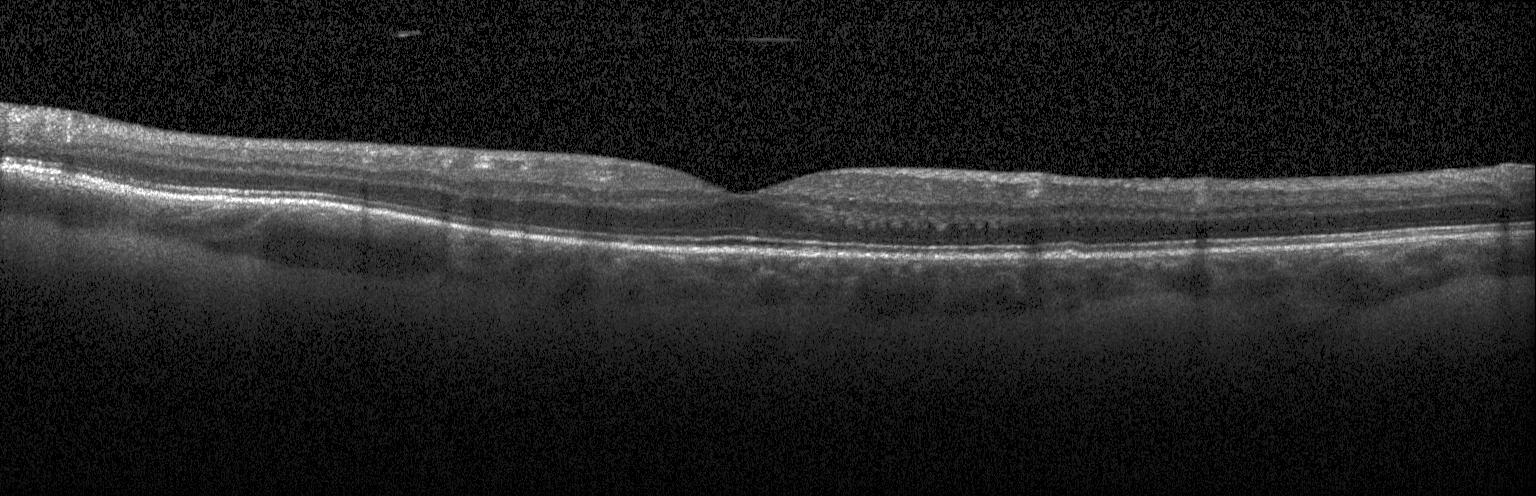 OCT line scan.
Macular OCT: no choroidal neovascularization, no diabetic macular edema, and no drusen.